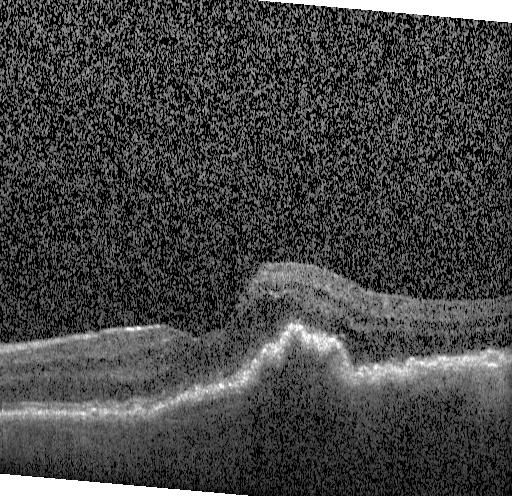
Finding: a choroidal neovascular membrane.